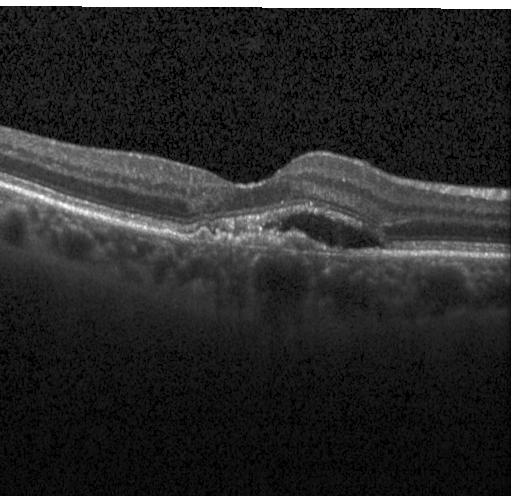
Impression: a choroidal neovascular membrane.